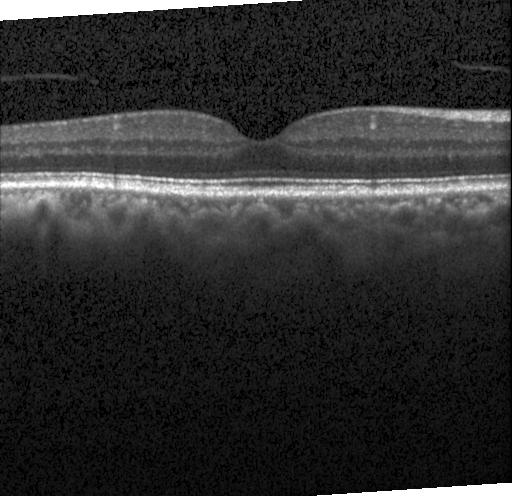 Horizontal scan through the fovea; optical coherence tomography B-scan; Heidelberg Spectralis
Macular OCT: no evidence of choroidal neovascularization, diabetic macular edema, or drusen.